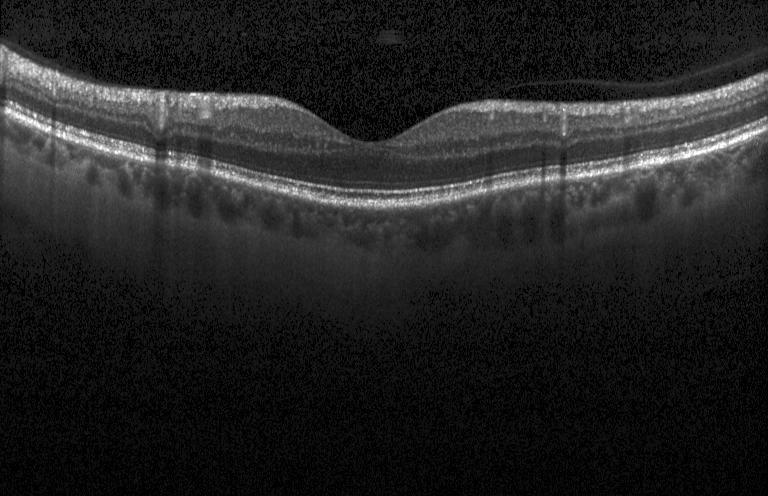 Spectral-domain optical coherence tomography. Centered on the fovea. Heidelberg Spectralis. OCT B-scan
Dx: neither choroidal neovascularization, diabetic macular edema, nor drusen.